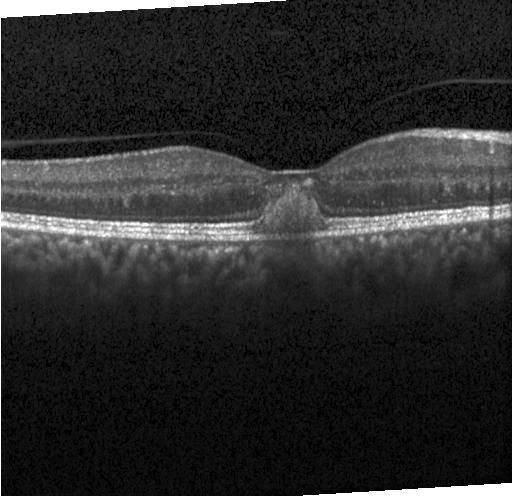 This B-scan demonstrates a choroidal neovascular membrane.